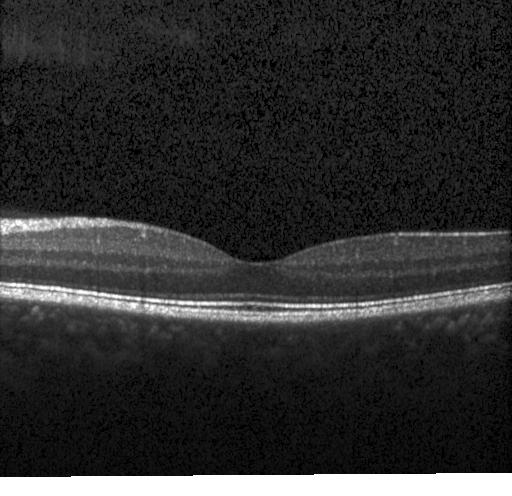

Optical coherence tomography B-scan · Heidelberg Spectralis. The scan shows no evidence of choroidal neovascularization, diabetic macular edema, or drusen.